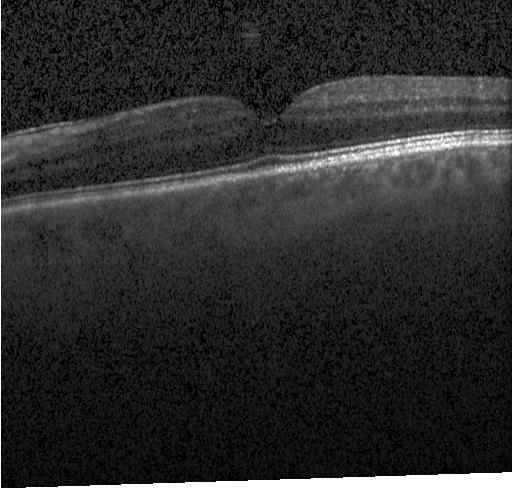
Retinal OCT B-scan; spectral-domain optical coherence tomography. No CNV, DME, or drusen.